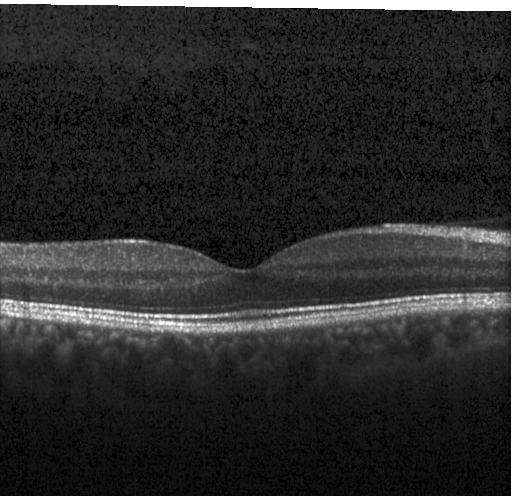
The scan shows no choroidal neovascularization, no diabetic macular edema, and no drusen.